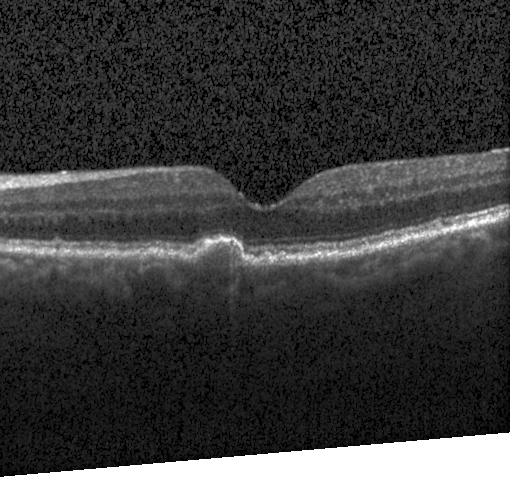

Retinal OCT cross-section; through the macula; SD-OCT. Dx: multiple drusen.